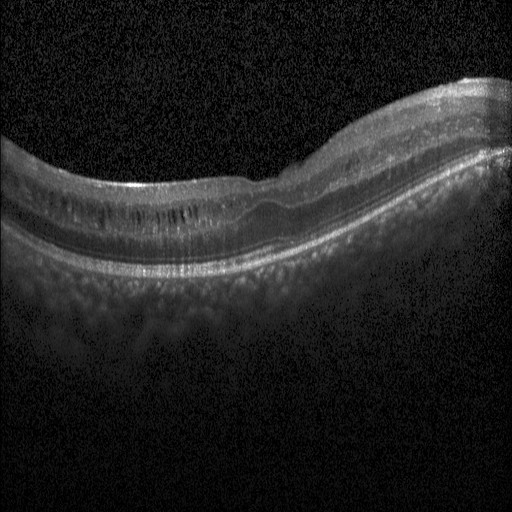 Macular OCT demonstrating diabetic macular edema (DME).